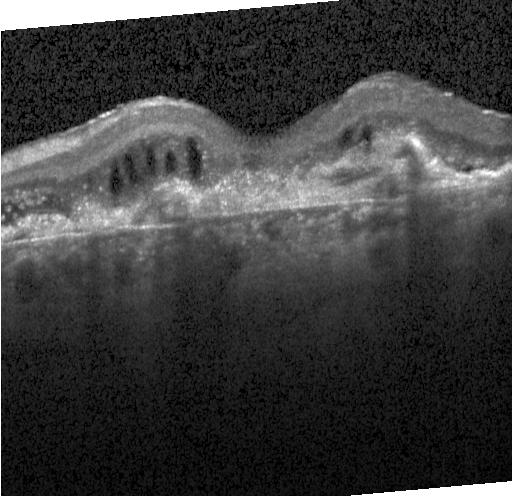

This B-scan demonstrates a choroidal neovascular membrane.